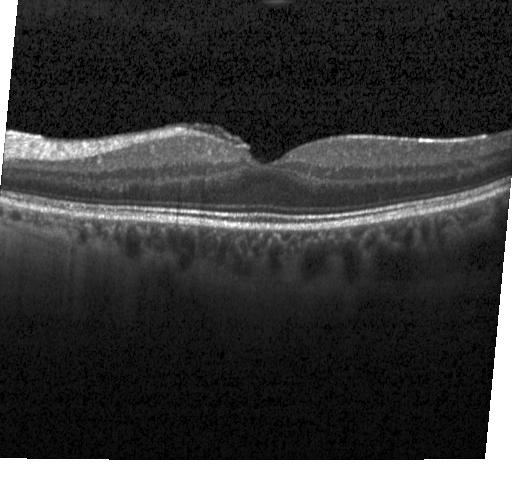 Macular OCT: no evidence of choroidal neovascularization, diabetic macular edema, or drusen.